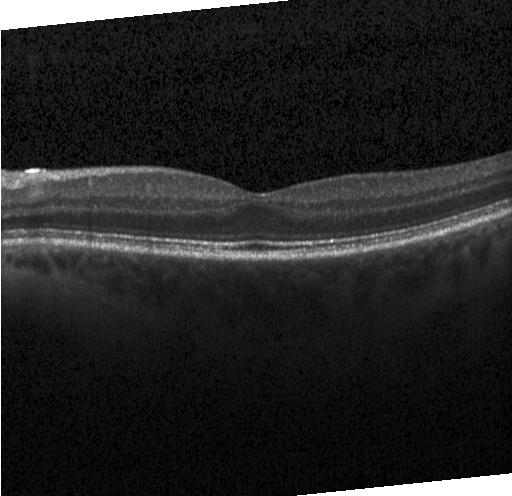 SD-OCT, through the macula, retinal OCT B-scan.
Diagnosis: no choroidal neovascularization, diabetic macular edema, or drusen.